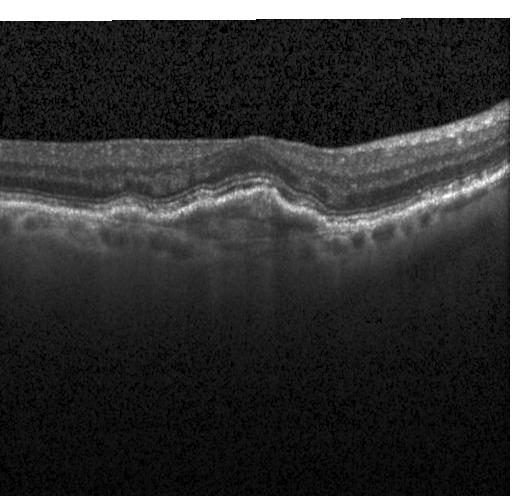 Retinal OCT B-scan. Macular OCT: CNV.